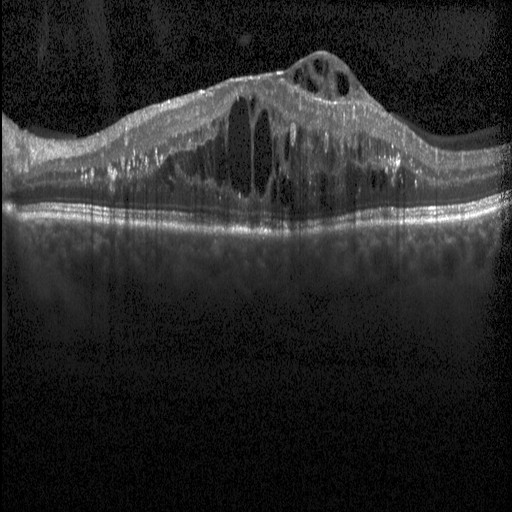 Finding: diabetic macular edema.